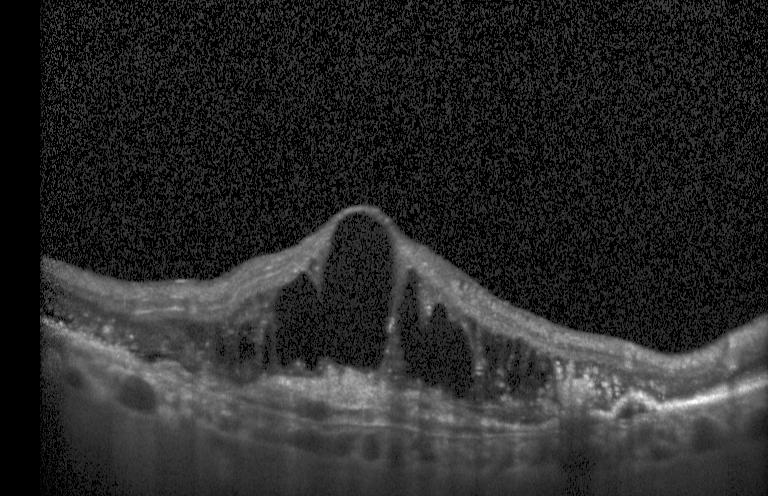 Retinal OCT cross-section
The scan shows a choroidal neovascular membrane.